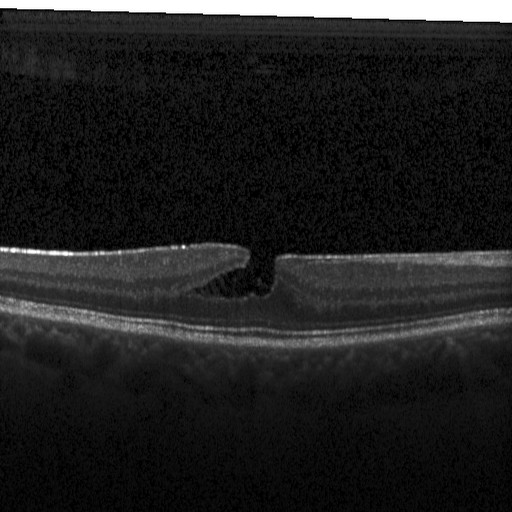
Retinal OCT cross-section showing diabetic macular edema.